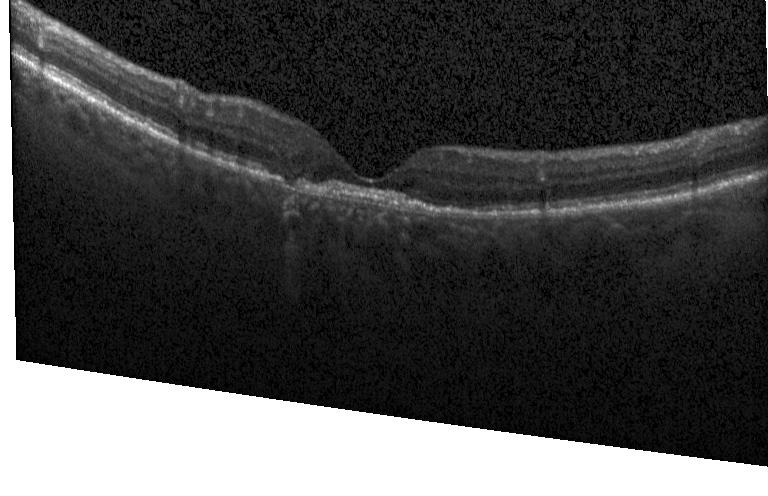 Retinal OCT cross-section. Spectral-domain OCT. Horizontal scan through the fovea. Heidelberg Spectralis. Dx: choroidal neovascularization.